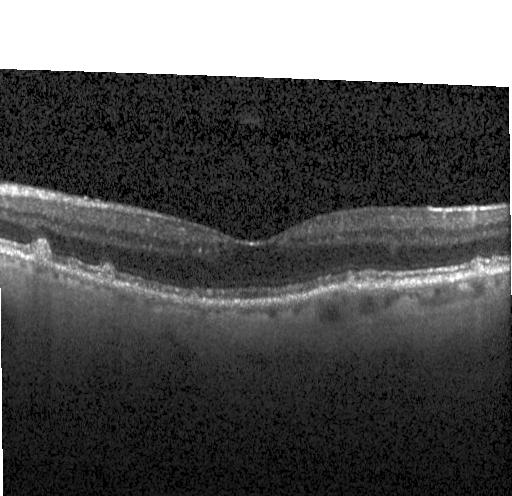

Optical coherence tomography B-scan · centered on the fovea · spectral-domain OCT
The scan shows drusen.